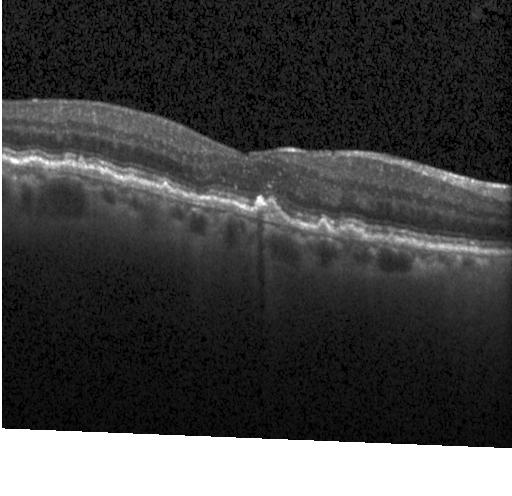 Finding: drusen.